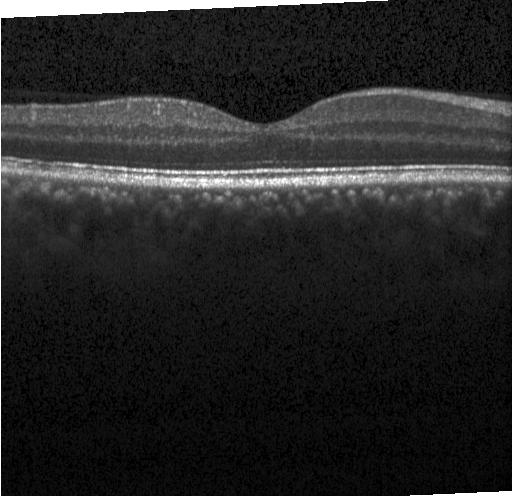

Optical coherence tomography B-scan · through the macula · Heidelberg Spectralis — Diagnosis: neither CNV, DME, nor drusen.